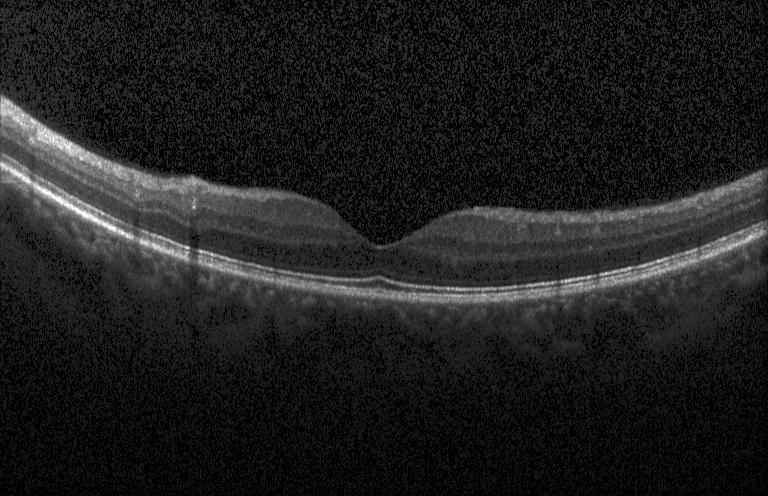

Finding: no CNV, no DME, and no drusen.